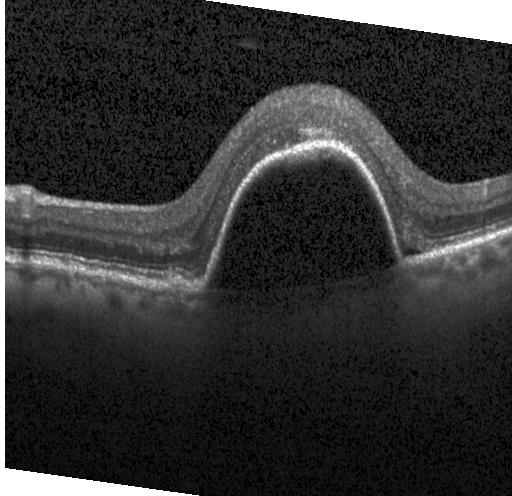 Retinal OCT B-scan · spectral-domain optical coherence tomography.
The scan shows choroidal neovascularization.